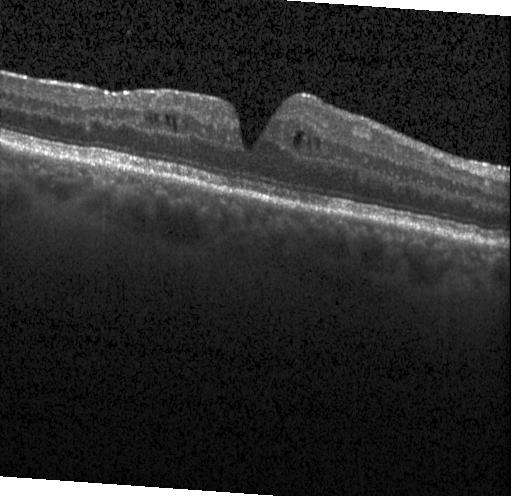

Instrument: Heidelberg Spectralis. Fovea-centered. Optical coherence tomography scan — Diagnosis: diabetic macular edema (DME).